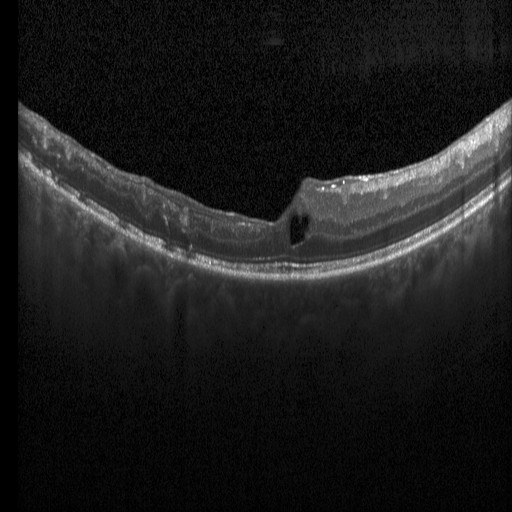

Acquired on a Heidelberg Spectralis. Retinal OCT cross-section. Macular scan.
Diabetic macular edema (DME).